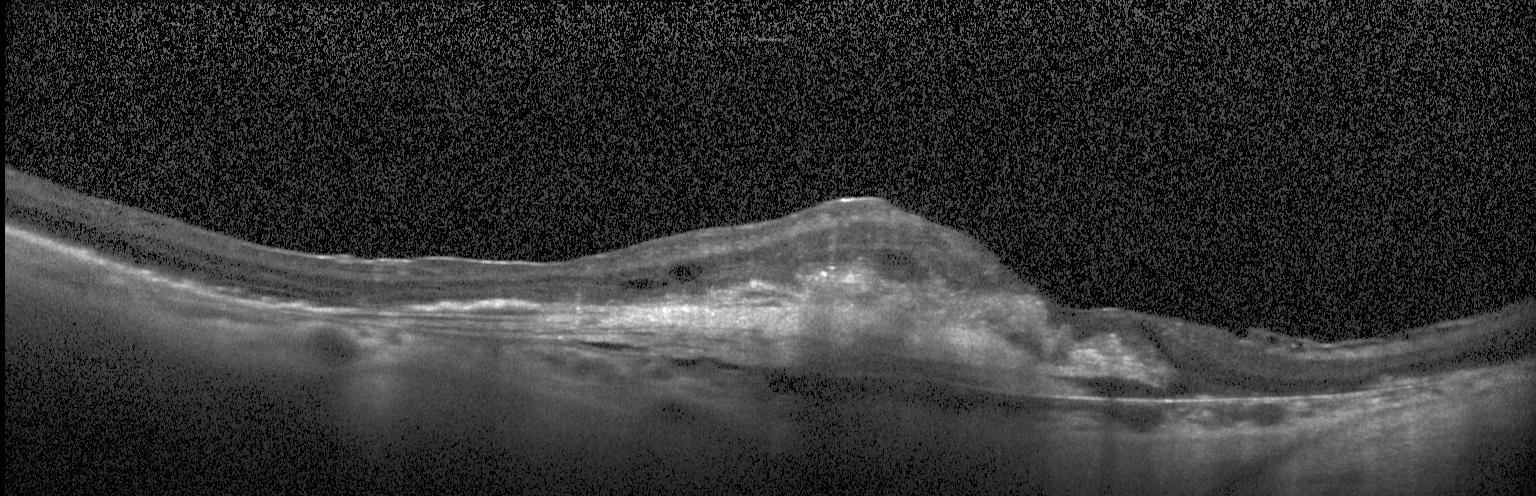 Retinal OCT cross-section showing a choroidal neovascular membrane.